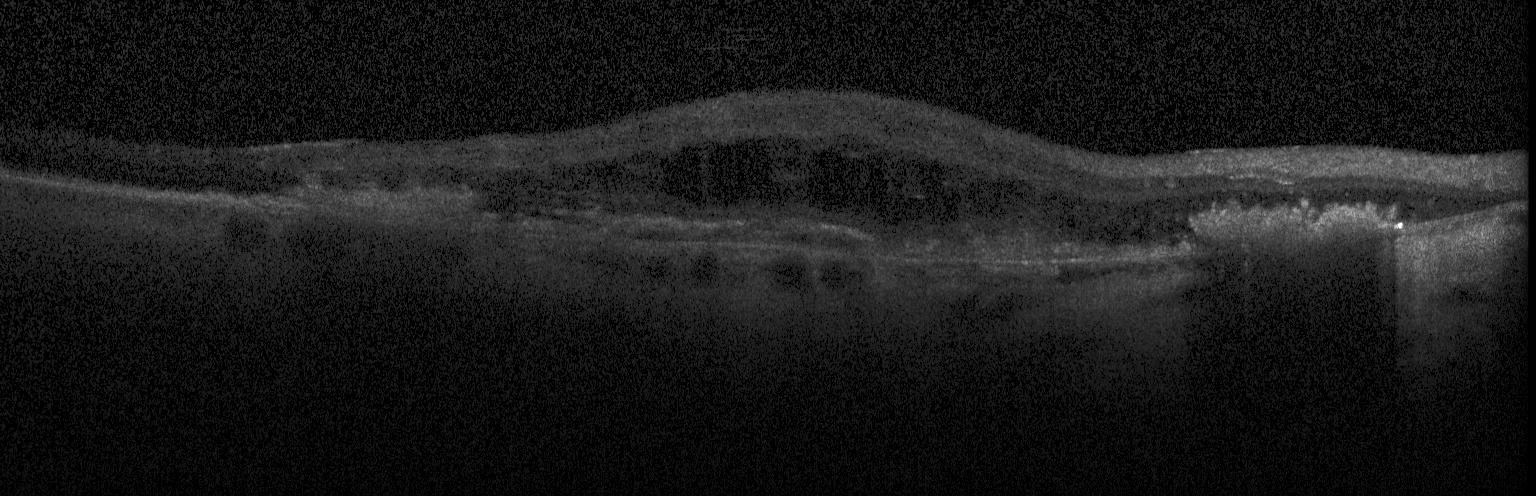

Spectral-domain optical coherence tomography; through the macula; optical coherence tomography B-scan; instrument: Heidelberg Spectralis — A choroidal neovascular membrane.